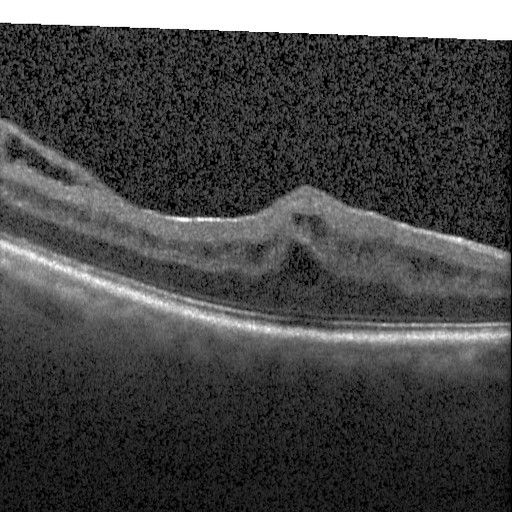 SD-OCT. Centered on the fovea. Retinal OCT B-scan
Dx: DME.